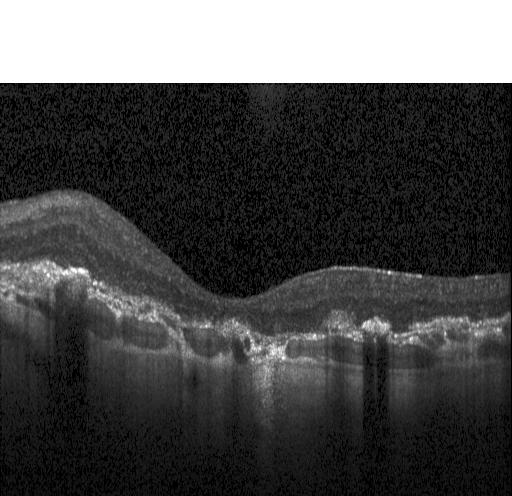 Spectral-domain OCT · OCT B-scan
Macular OCT: choroidal neovascularization.